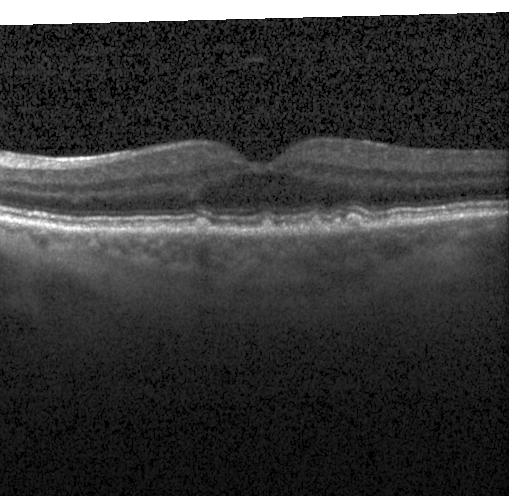

SD-OCT · horizontal scan through the fovea · OCT B-scan. Sub-RPE drusenoid deposits.